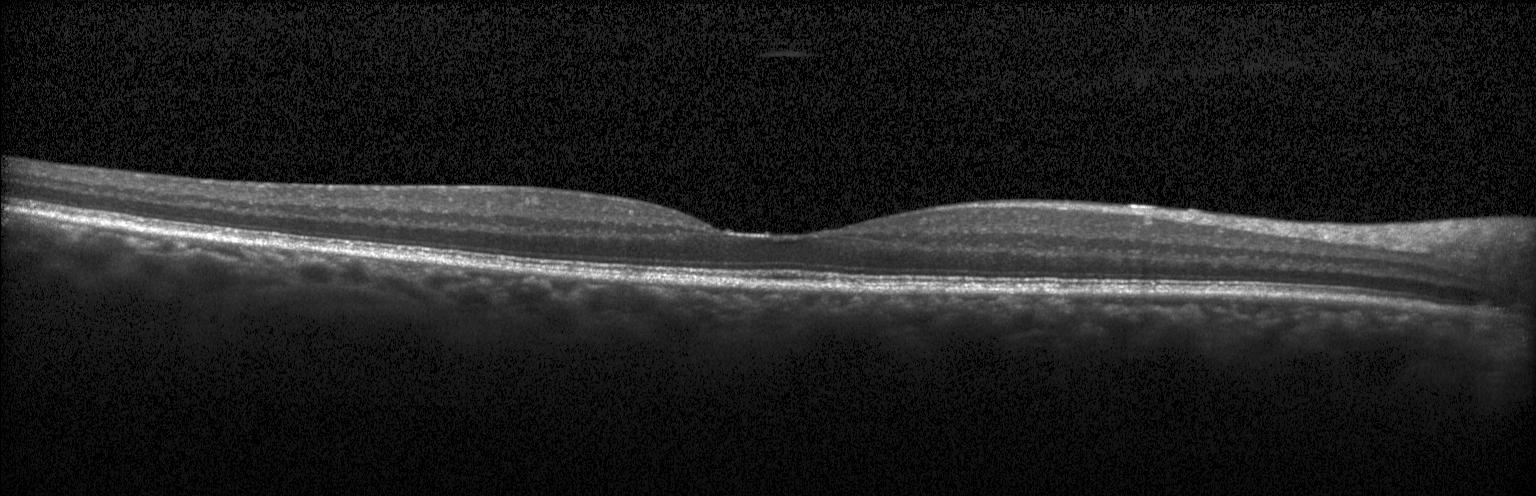 Spectral-domain optical coherence tomography · acquired on a Heidelberg Spectralis · OCT line scan. Diagnosis: no choroidal neovascularization, no diabetic macular edema, and no drusen.